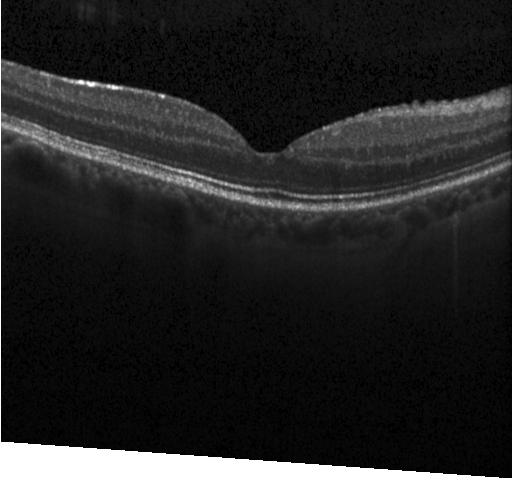 Retinal OCT B-scan; acquired on a Heidelberg Spectralis; macular scan
The scan shows no evidence of choroidal neovascularization, diabetic macular edema, or drusen.